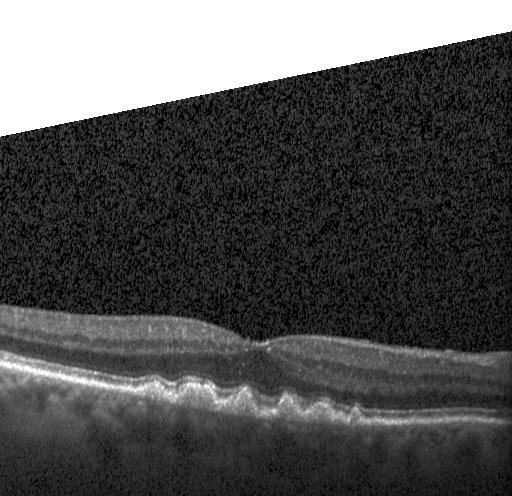
Optical coherence tomography scan.
Assessment: multiple drusen.